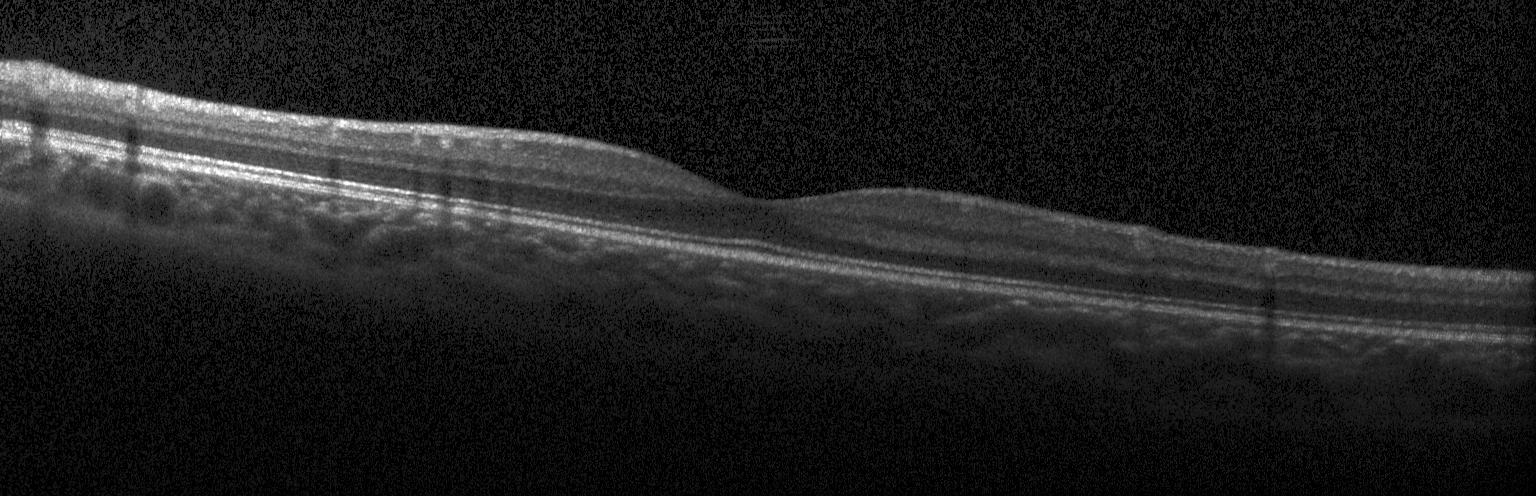
Fovea-centered. OCT line scan.
Diagnosis: neither CNV, DME, nor drusen.